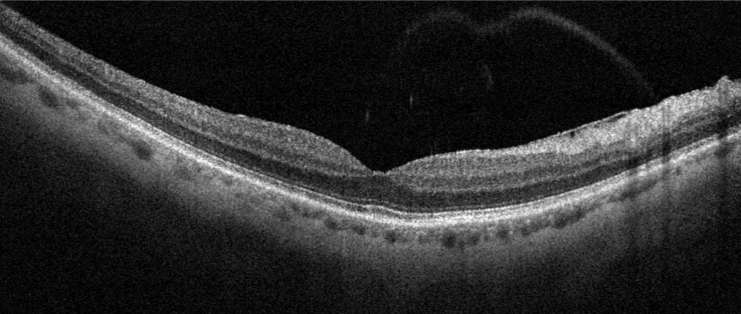
Diagnosis: epiretinal membrane (ERM).